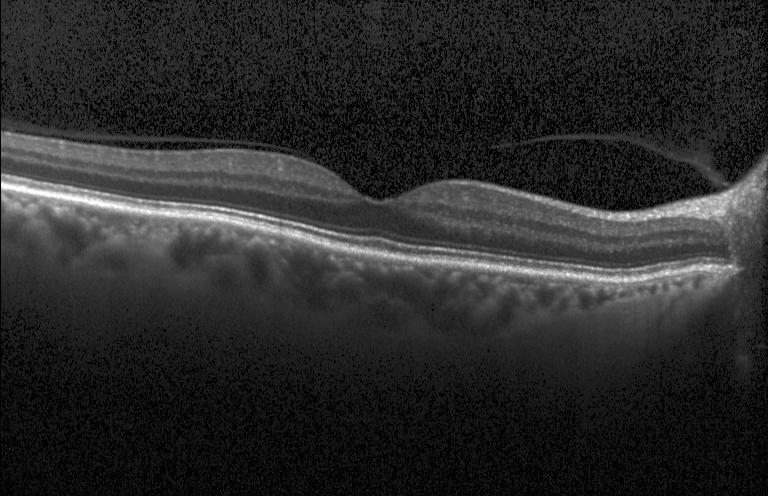

Optical coherence tomography scan — Impression: no choroidal neovascularization, no diabetic macular edema, and no drusen.